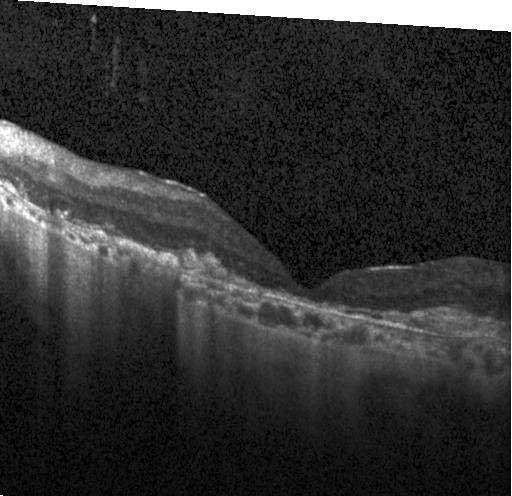

CNV.